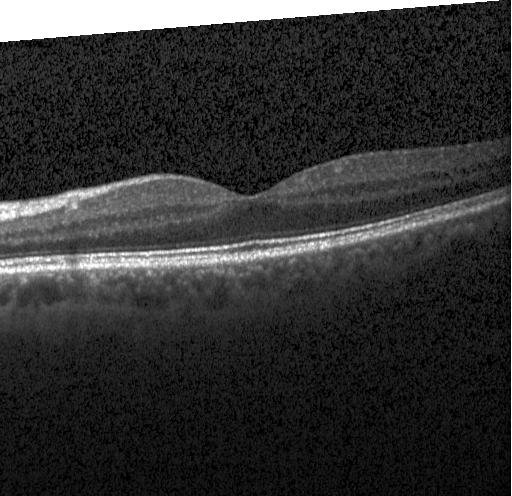 OCT B-scan
Neither choroidal neovascularization, diabetic macular edema, nor drusen.